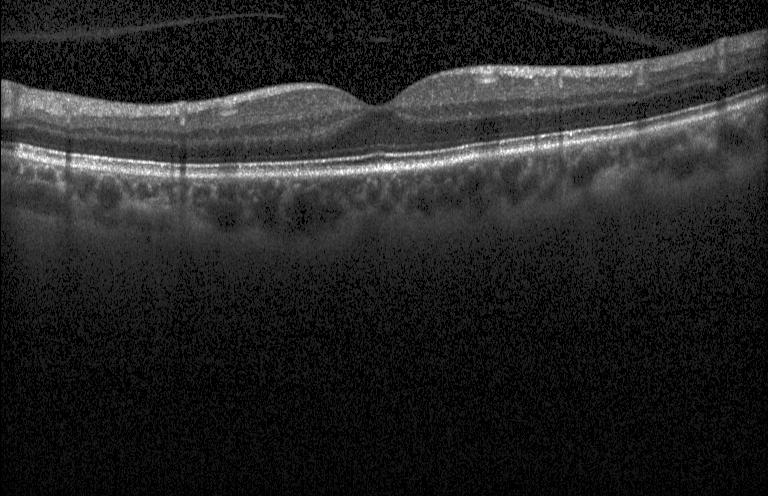 Macular OCT demonstrating no evidence of CNV, DME, or drusen.